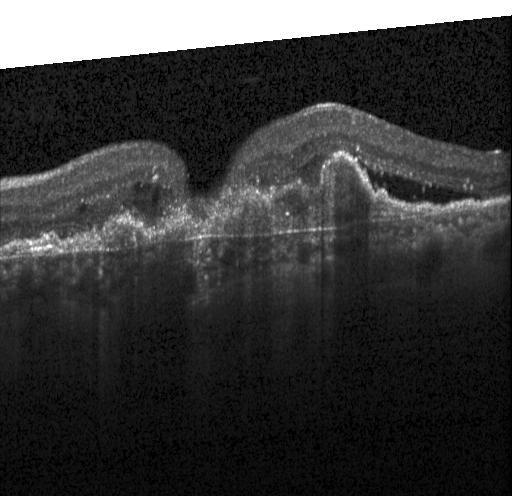
Finding: CNV.